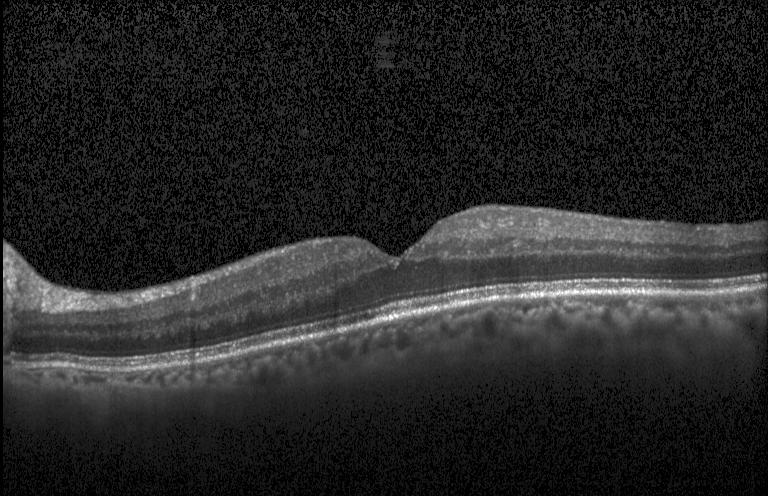 Impression: no CNV, DME, or drusen.